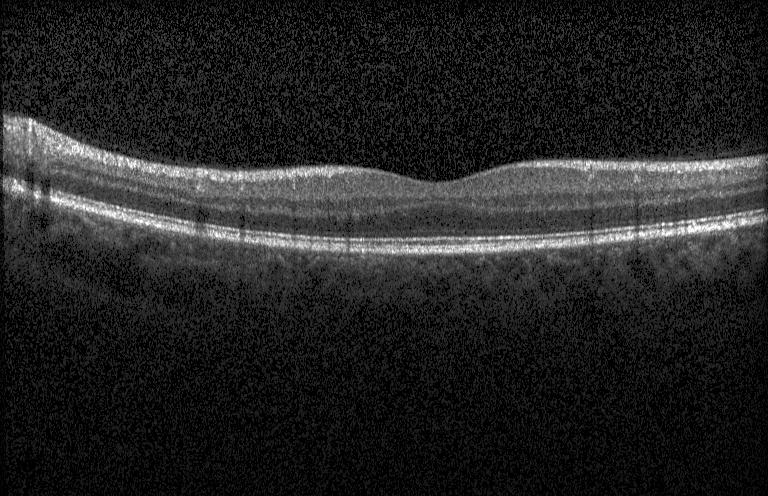 OCT finding: neither choroidal neovascularization, diabetic macular edema, nor drusen.